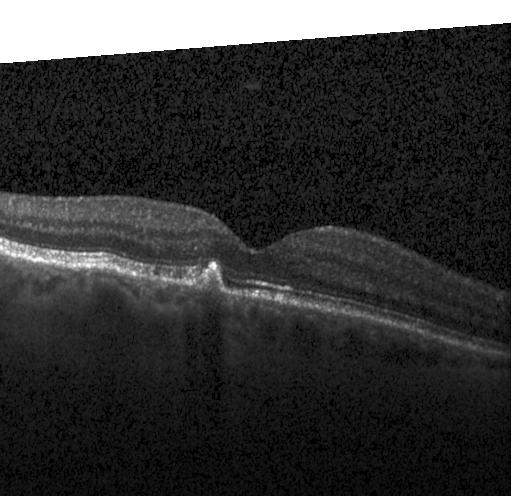 Impression: multiple drusen.